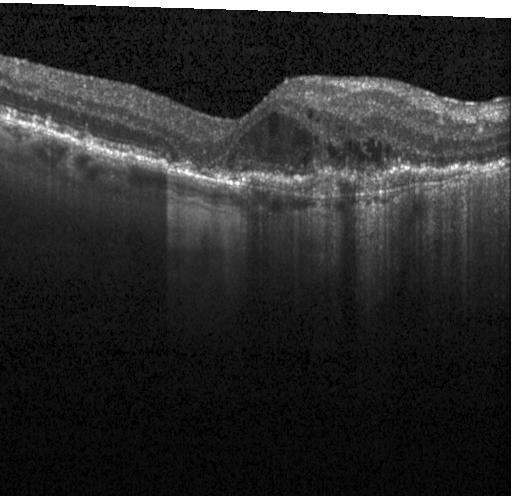 Optical coherence tomography B-scan. Through the macula — Finding: a choroidal neovascular membrane.